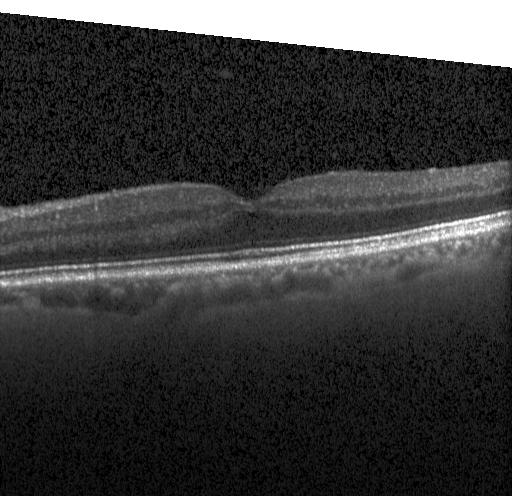
OCT B-scan · Heidelberg Spectralis · spectral-domain OCT.
The scan shows neither CNV, DME, nor drusen.